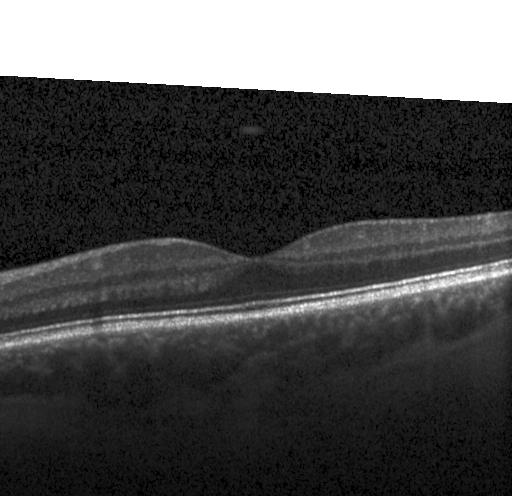 OCT line scan — Finding: no choroidal neovascularization, no diabetic macular edema, and no drusen.